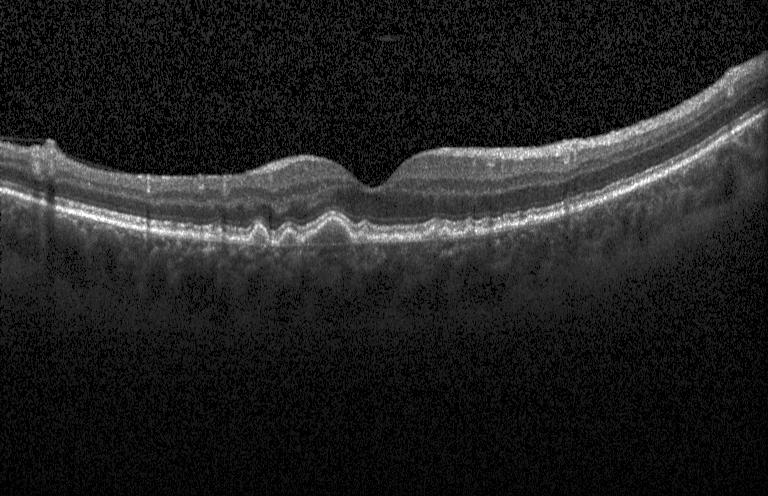 SD-OCT; retinal OCT B-scan — Finding: drusen.